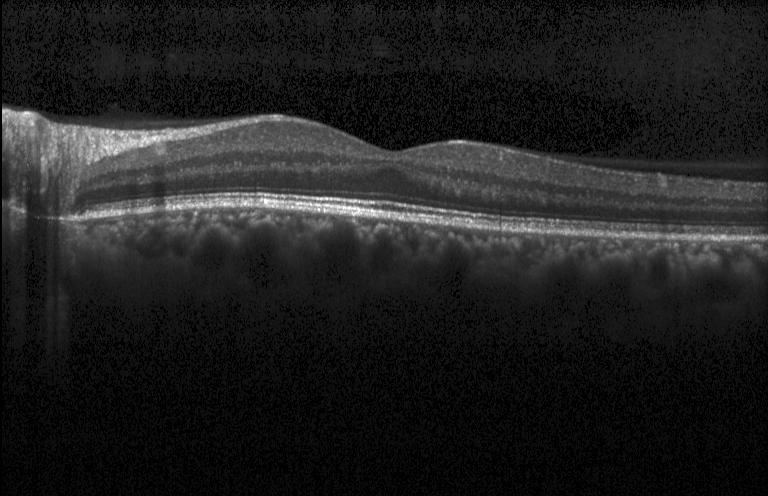 Retinal OCT B-scan, acquired on a Heidelberg Spectralis, spectral-domain OCT.
Dx: no CNV, DME, or drusen.